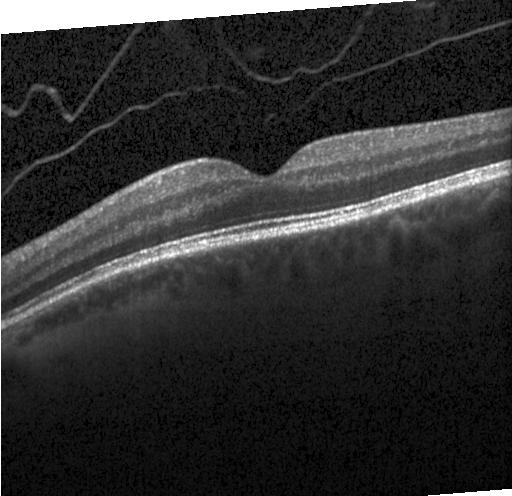
Retinal OCT cross-section, spectral-domain OCT, through the macula.
Macular OCT: no choroidal neovascularization, no diabetic macular edema, and no drusen.